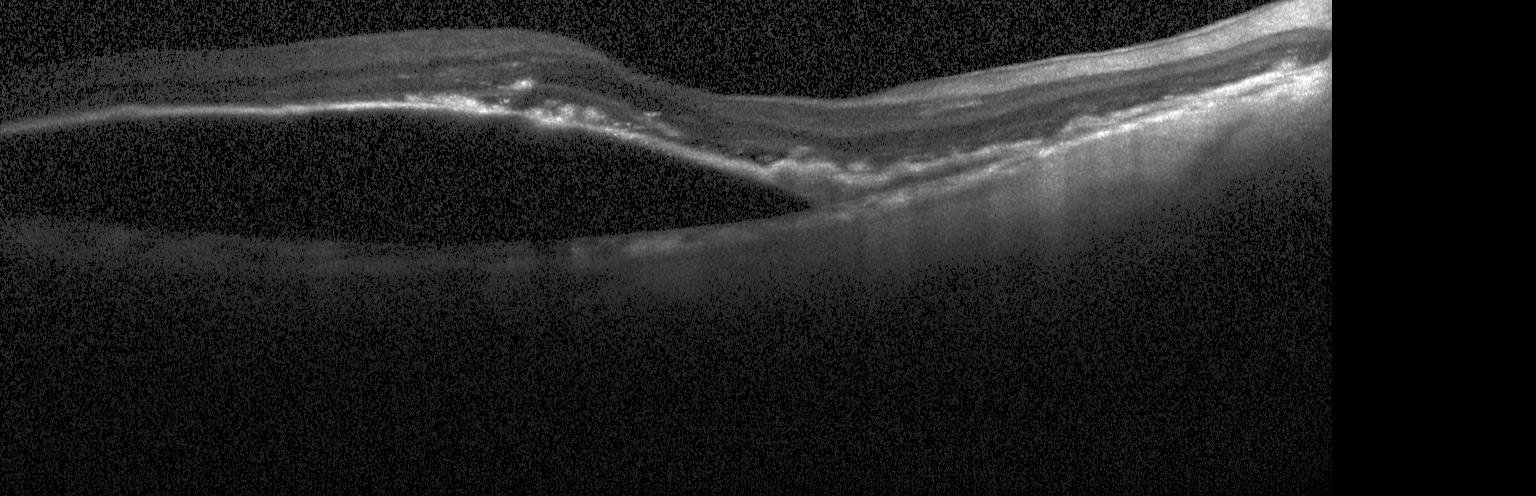 Assessment: a choroidal neovascular membrane.